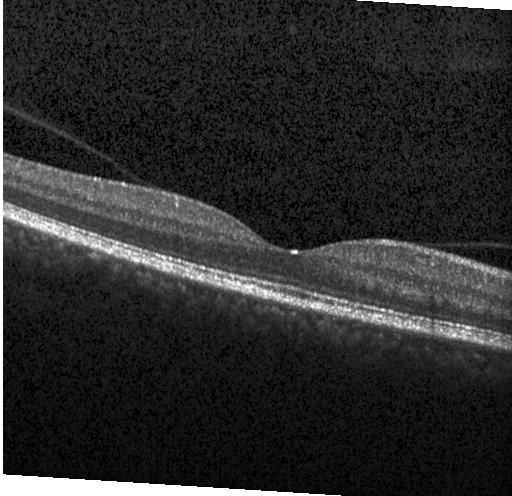

Macular OCT: no choroidal neovascularization, no diabetic macular edema, and no drusen.